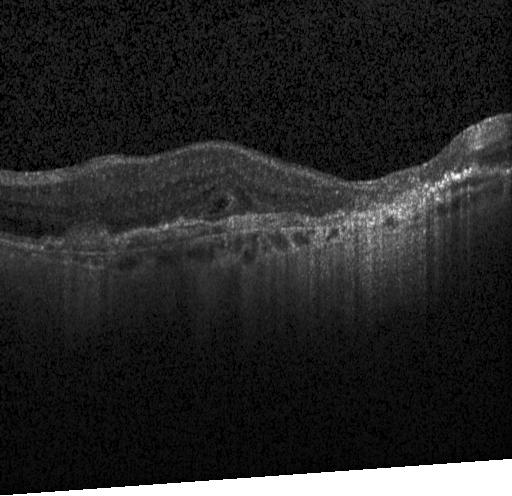
OCT B-scan showing CNV.